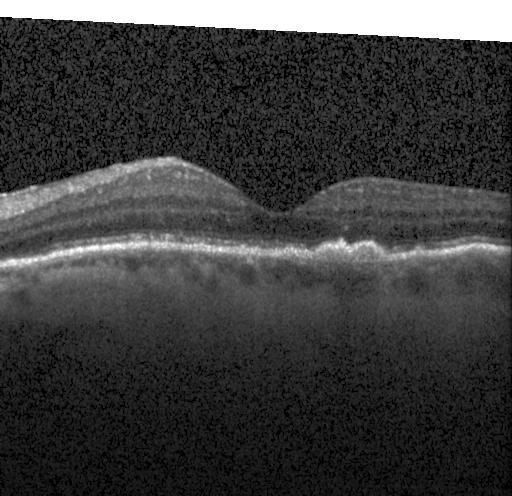 Spectral-domain optical coherence tomography · OCT line scan · horizontal scan through the fovea · instrument: Heidelberg Spectralis — Impression: a choroidal neovascular membrane.